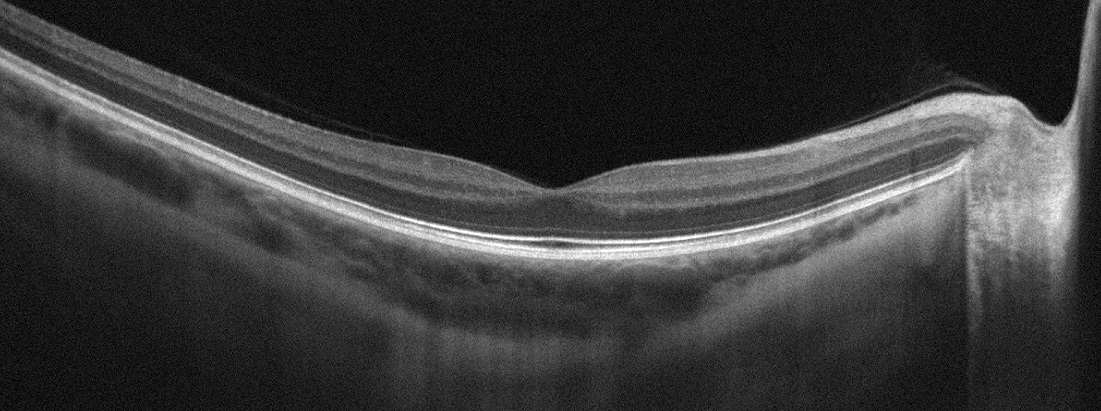

OCT line scan.
The scan shows no evidence of AMD, DME, ERM, RAO, RVO, or VID.